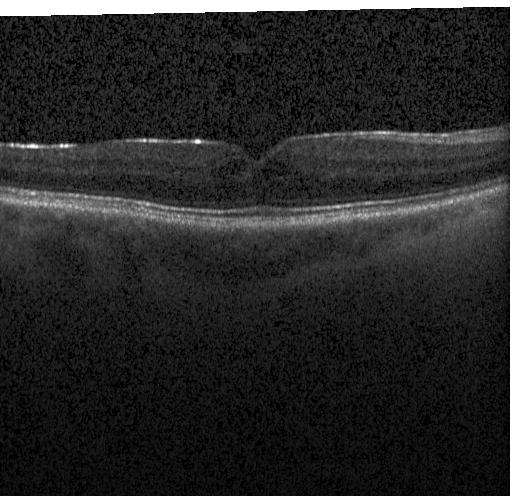 Heidelberg Spectralis OCT system, fovea-centered, spectral-domain optical coherence tomography, OCT B-scan — This B-scan demonstrates DME.